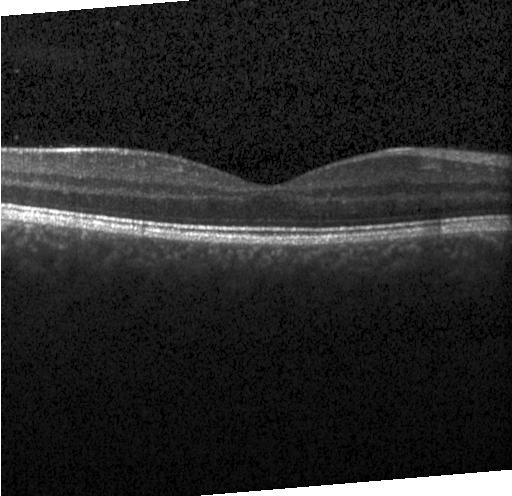

Retinal OCT cross-section · spectral-domain OCT · macular scan. Impression: neither CNV, DME, nor drusen.